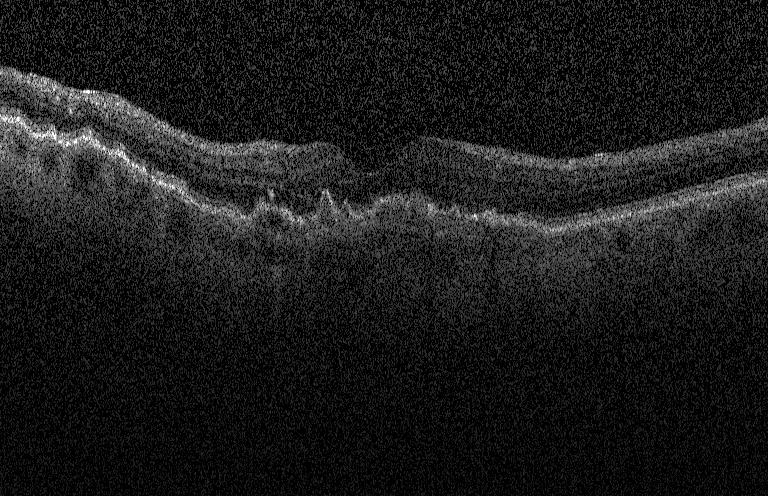
OCT finding: choroidal neovascularization.